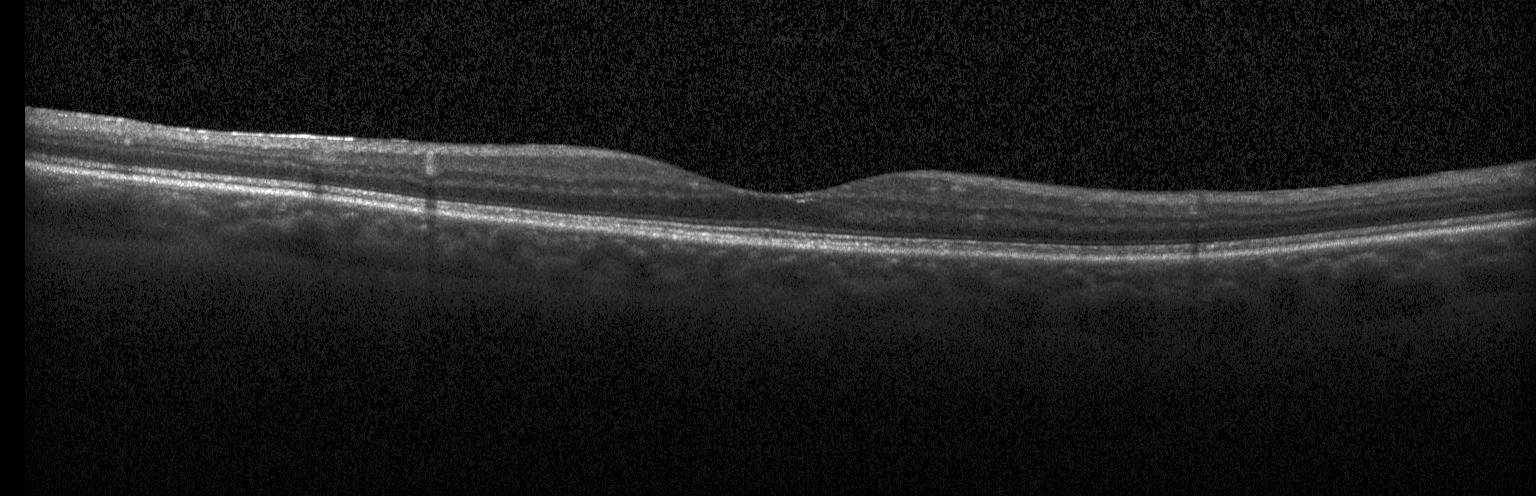 Optical coherence tomography scan
OCT finding: neither choroidal neovascularization, diabetic macular edema, nor drusen.